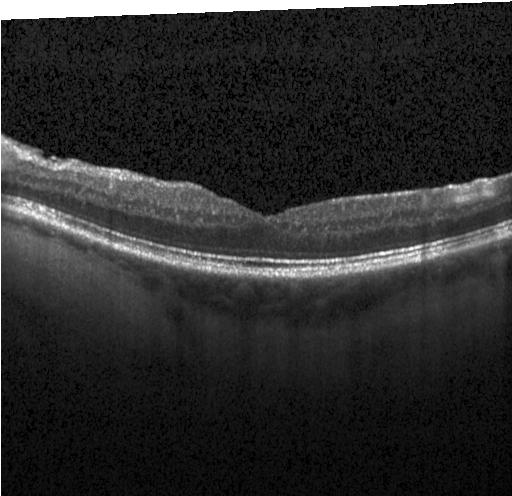
OCT B-scan; spectral-domain OCT; instrument: Heidelberg Spectralis.
OCT finding: neither choroidal neovascularization, diabetic macular edema, nor drusen.